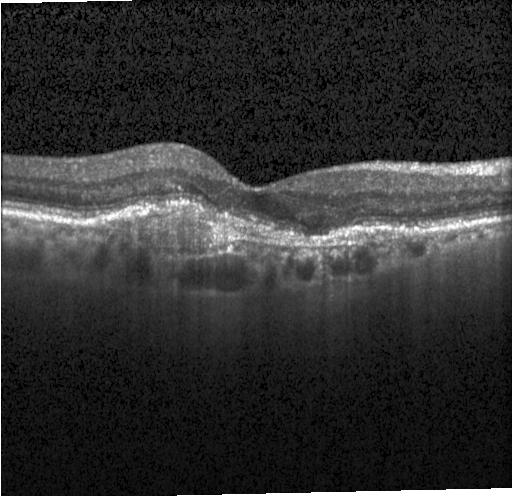
Optical coherence tomography B-scan · SD-OCT.
Assessment: a choroidal neovascular membrane.